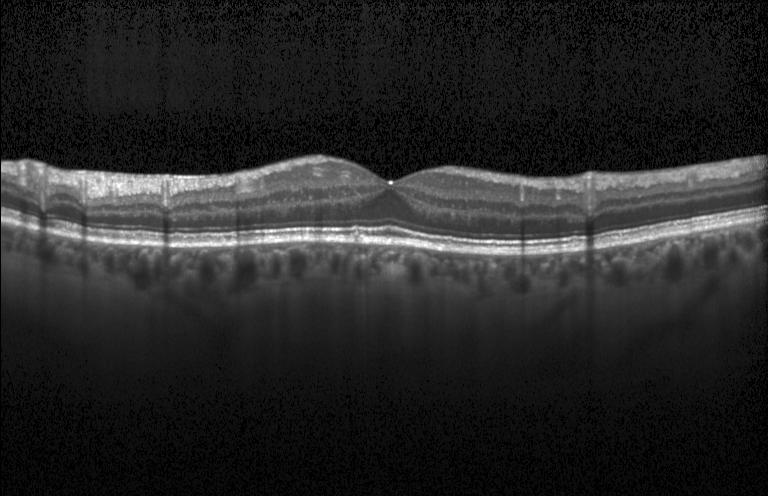 Heidelberg Spectralis, OCT B-scan.
Dx: sub-RPE drusenoid deposits.